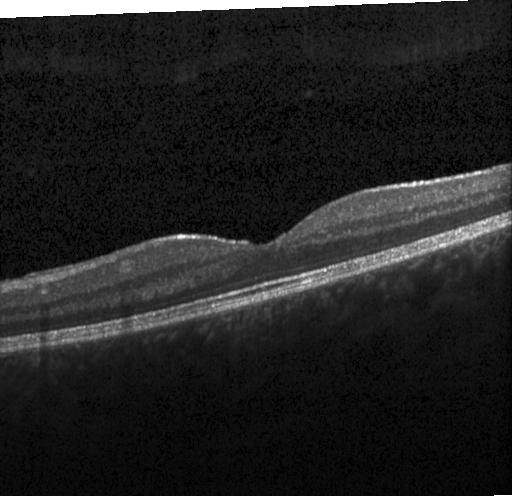

Spectral-domain OCT, optical coherence tomography scan. Finding: no evidence of choroidal neovascularization, diabetic macular edema, or drusen.